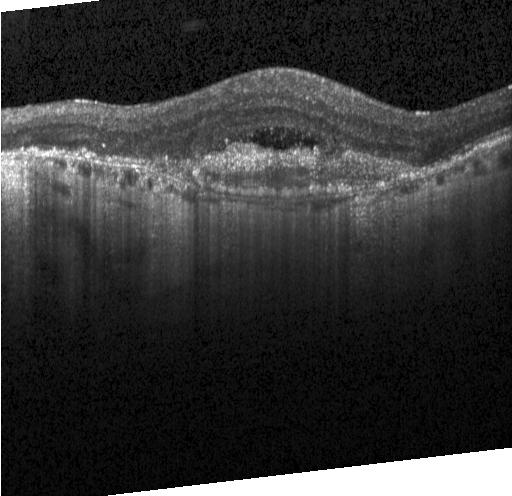

Retinal OCT B-scan, centered on the fovea
Impression: a choroidal neovascular membrane.